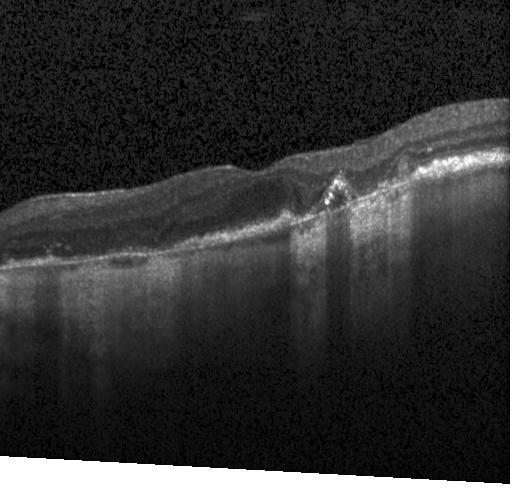

Instrument: Heidelberg Spectralis. Spectral-domain optical coherence tomography. Optical coherence tomography scan
Finding: CNV.